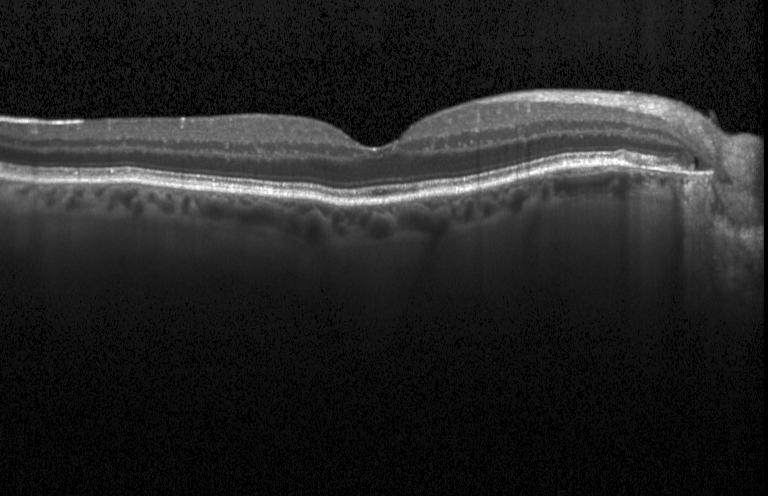 Optical coherence tomography scan; instrument: Heidelberg Spectralis; SD-OCT; macular scan. Impression: neither choroidal neovascularization, diabetic macular edema, nor drusen.